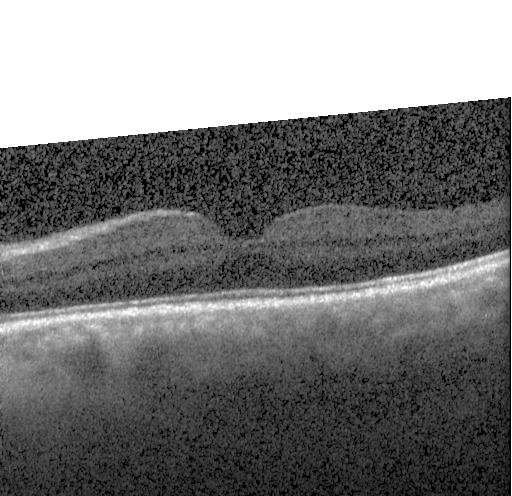
Spectral-domain OCT B-scan: no choroidal neovascularization, no diabetic macular edema, and no drusen.